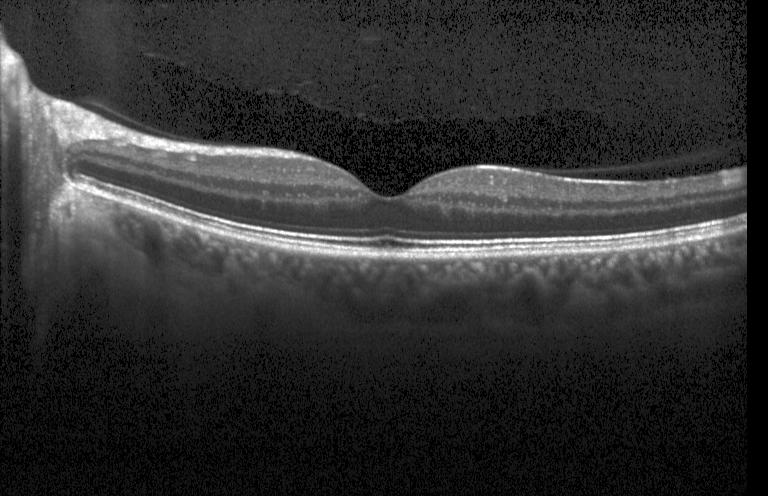
Retinal OCT B-scan.
OCT finding: neither CNV, DME, nor drusen.